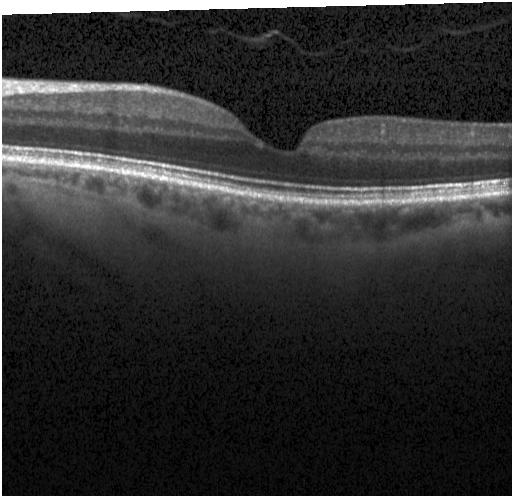

Retinal OCT B-scan; SD-OCT.
The scan shows no choroidal neovascularization, no diabetic macular edema, and no drusen.